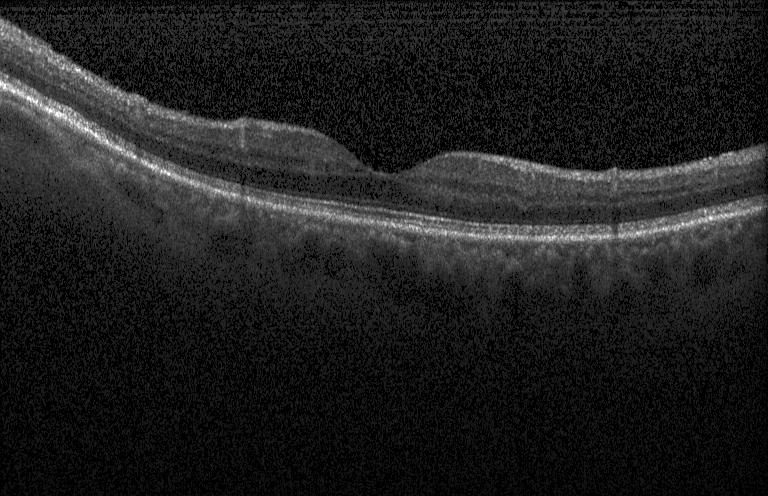 Dx: neither choroidal neovascularization, diabetic macular edema, nor drusen.